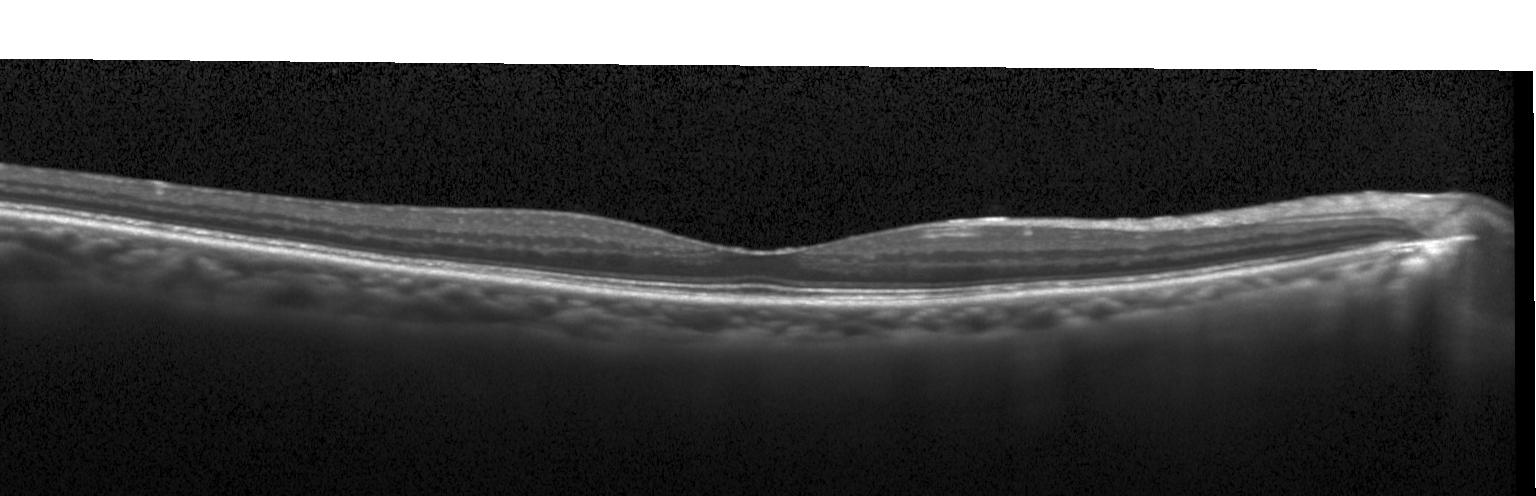 This B-scan demonstrates no CNV, no DME, and no drusen.